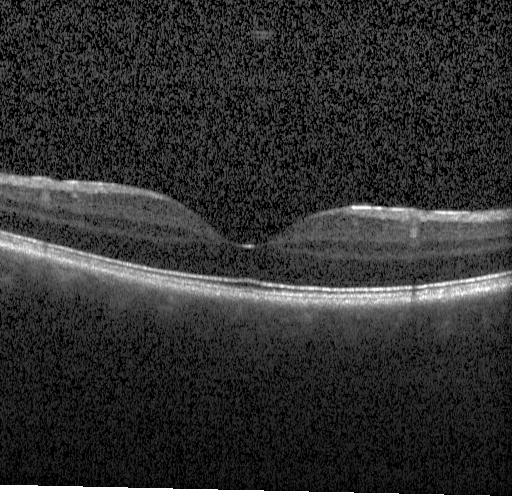

OCT B-scan.
Finding: neither CNV, DME, nor drusen.